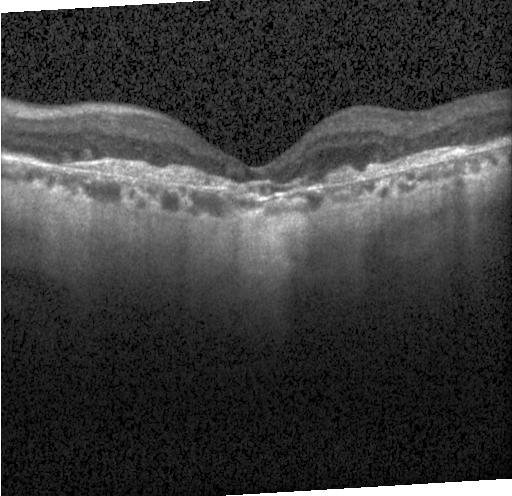

OCT finding: a choroidal neovascular membrane.